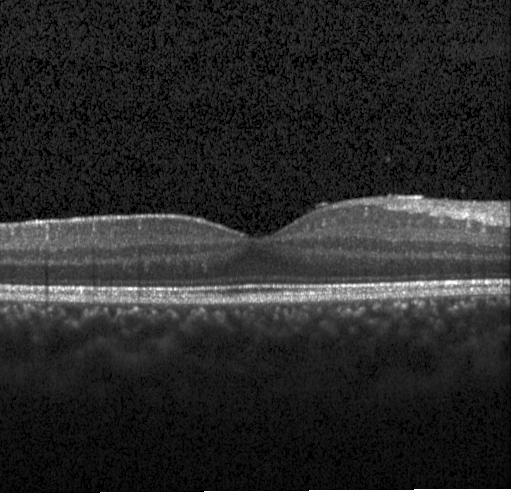
Fovea-centered; OCT line scan.
Impression: no choroidal neovascularization, diabetic macular edema, or drusen.